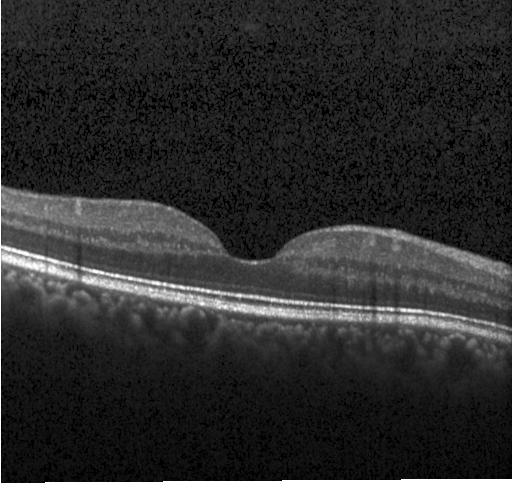 Heidelberg Spectralis; spectral-domain OCT; optical coherence tomography B-scan; macular scan — Diagnosis: neither choroidal neovascularization, diabetic macular edema, nor drusen.